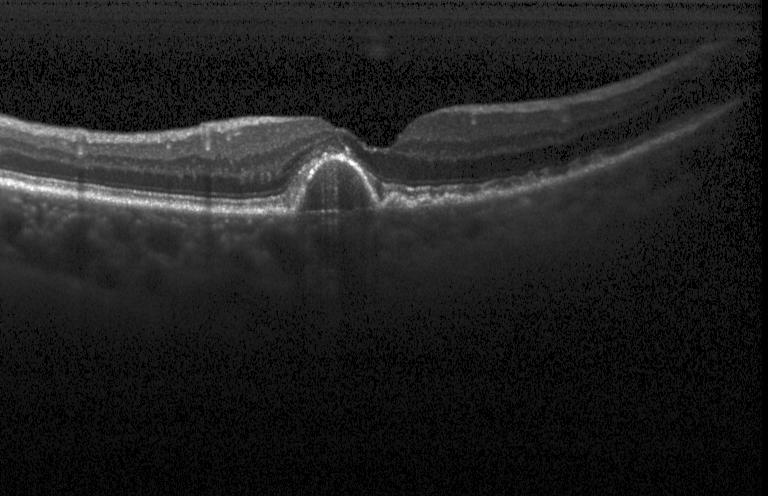 Through the macula. OCT B-scan — This B-scan demonstrates a choroidal neovascular membrane.